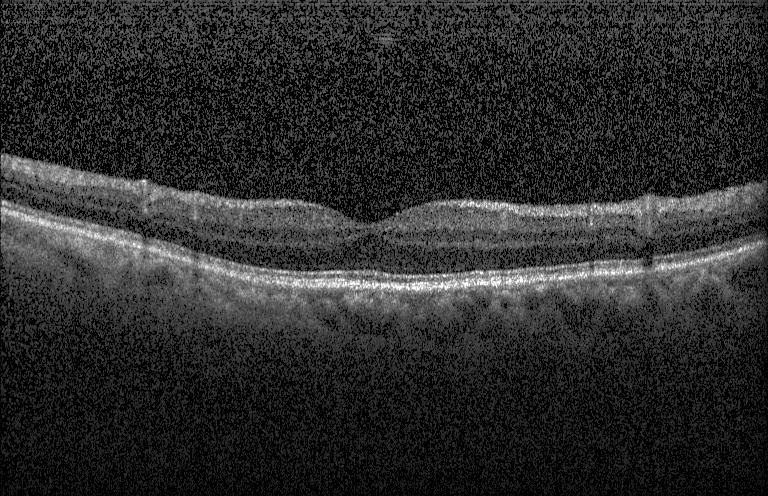
SD-OCT; centered on the fovea; optical coherence tomography B-scan; acquired on a Heidelberg Spectralis.
Impression: no CNV, no DME, and no drusen.